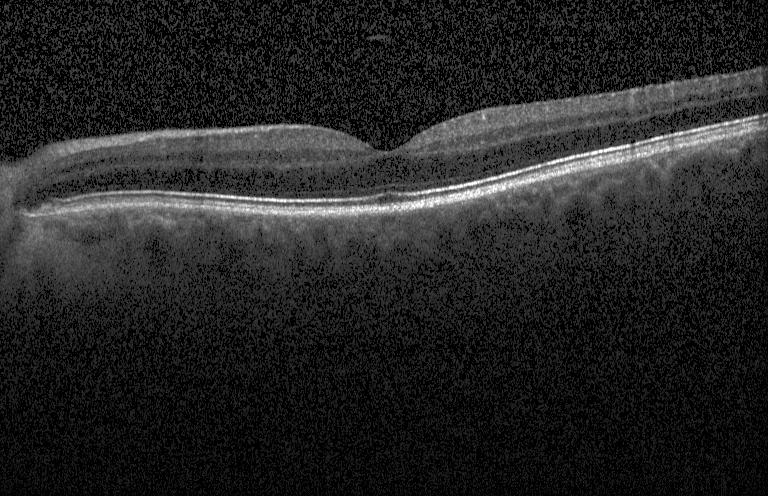
Retinal OCT cross-section — Impression: no evidence of choroidal neovascularization, diabetic macular edema, or drusen.